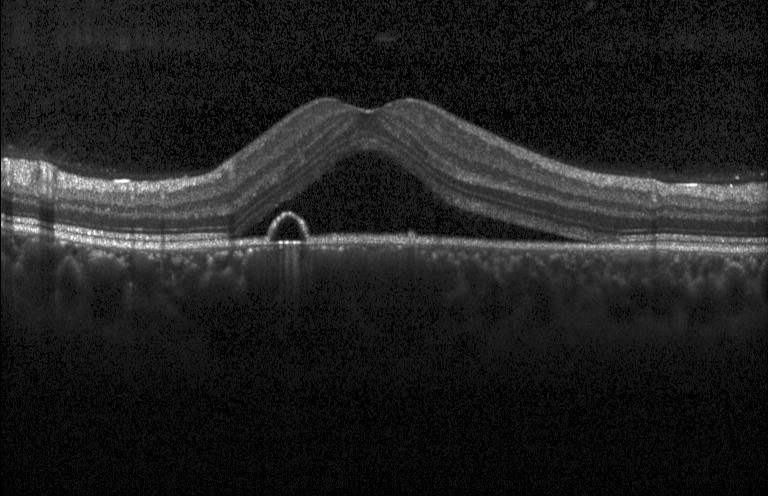
The scan shows a choroidal neovascular membrane.